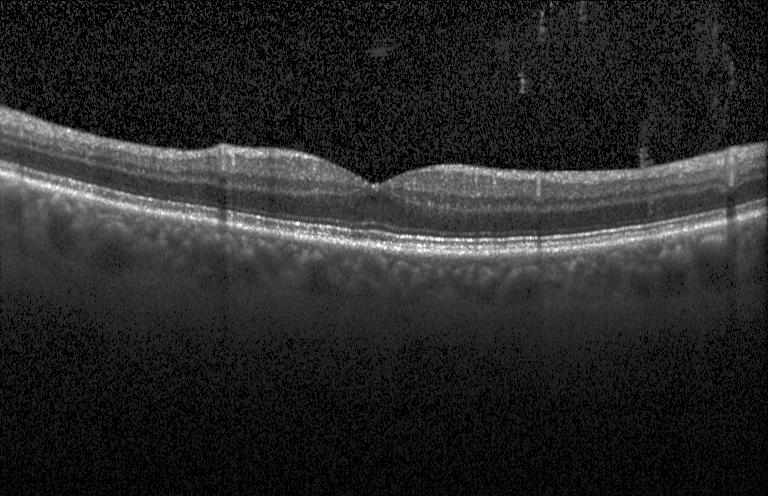
Horizontal scan through the fovea, retinal OCT B-scan, Heidelberg Spectralis, spectral-domain optical coherence tomography
Finding: no choroidal neovascularization, no diabetic macular edema, and no drusen.